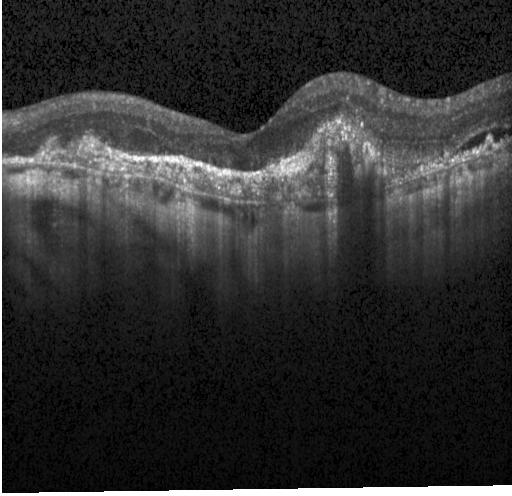

OCT line scan. Centered on the fovea — Diagnosis: CNV.